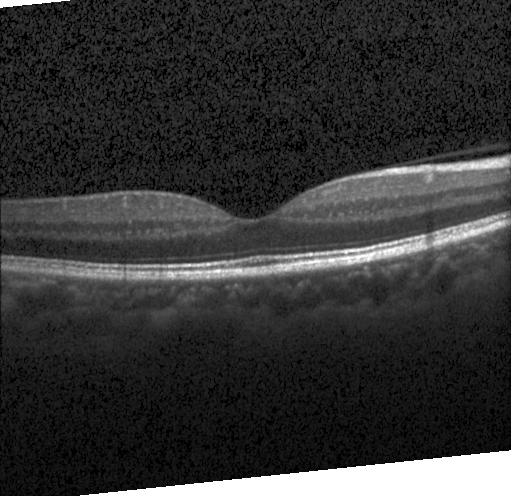

OCT line scan — Macular OCT: no evidence of choroidal neovascularization, diabetic macular edema, or drusen.